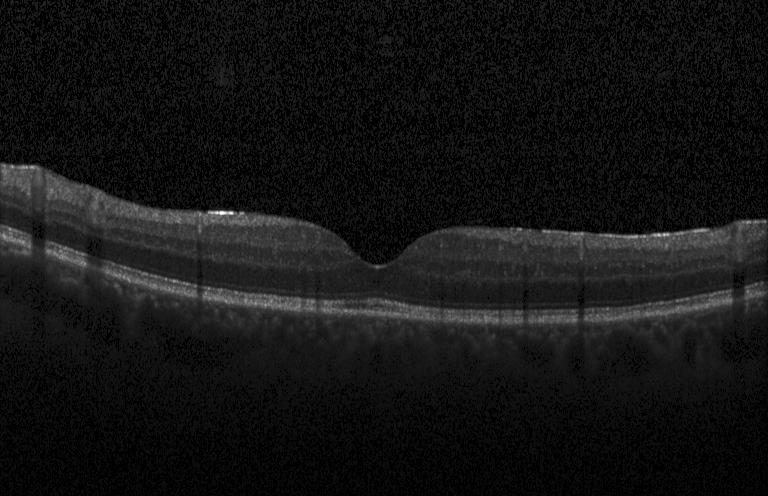

Retinal OCT cross-section showing no choroidal neovascularization, no diabetic macular edema, and no drusen.